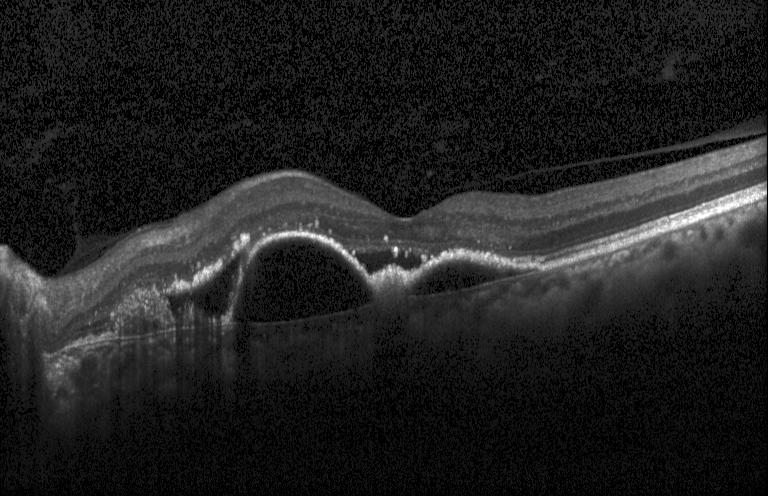

Diagnosis: CNV.